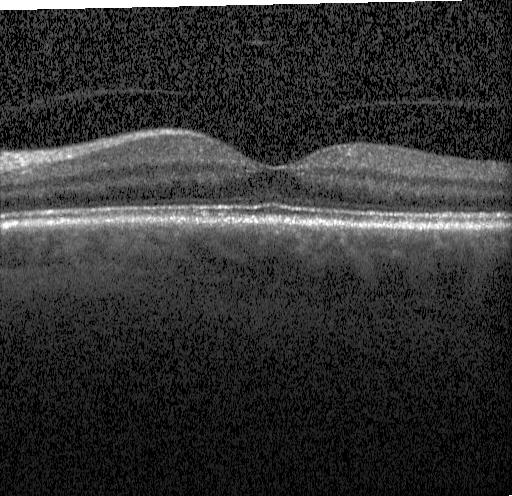
Heidelberg Spectralis · retinal OCT cross-section · spectral-domain optical coherence tomography — Diagnosis: no choroidal neovascularization, diabetic macular edema, or drusen.